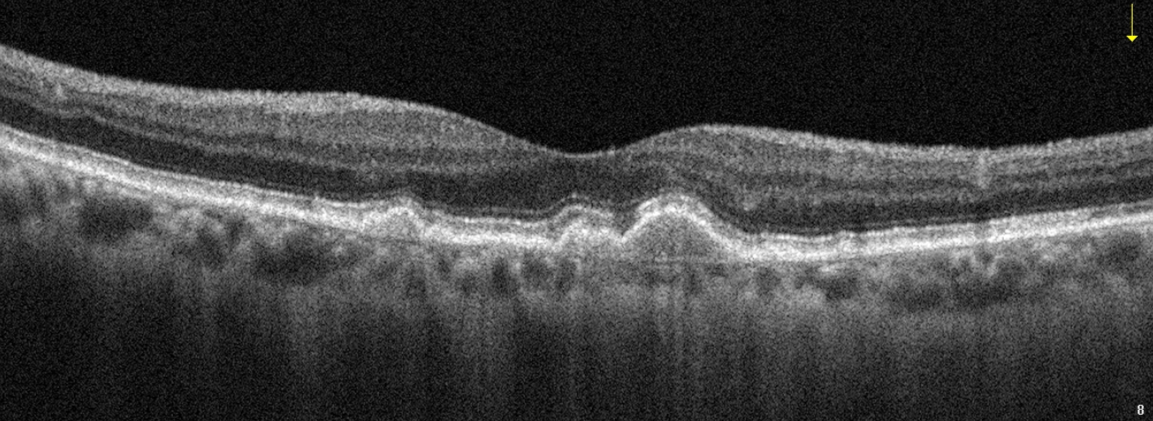

Optical coherence tomography B-scan
Diagnosis: AMD.